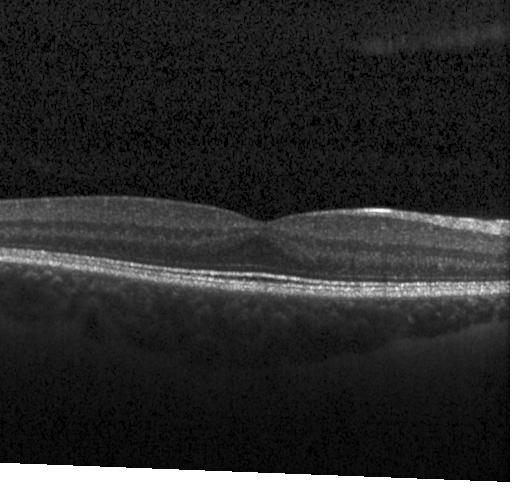

OCT line scan, through the macula, spectral-domain optical coherence tomography, instrument: Heidelberg Spectralis — The scan shows no choroidal neovascularization, no diabetic macular edema, and no drusen.